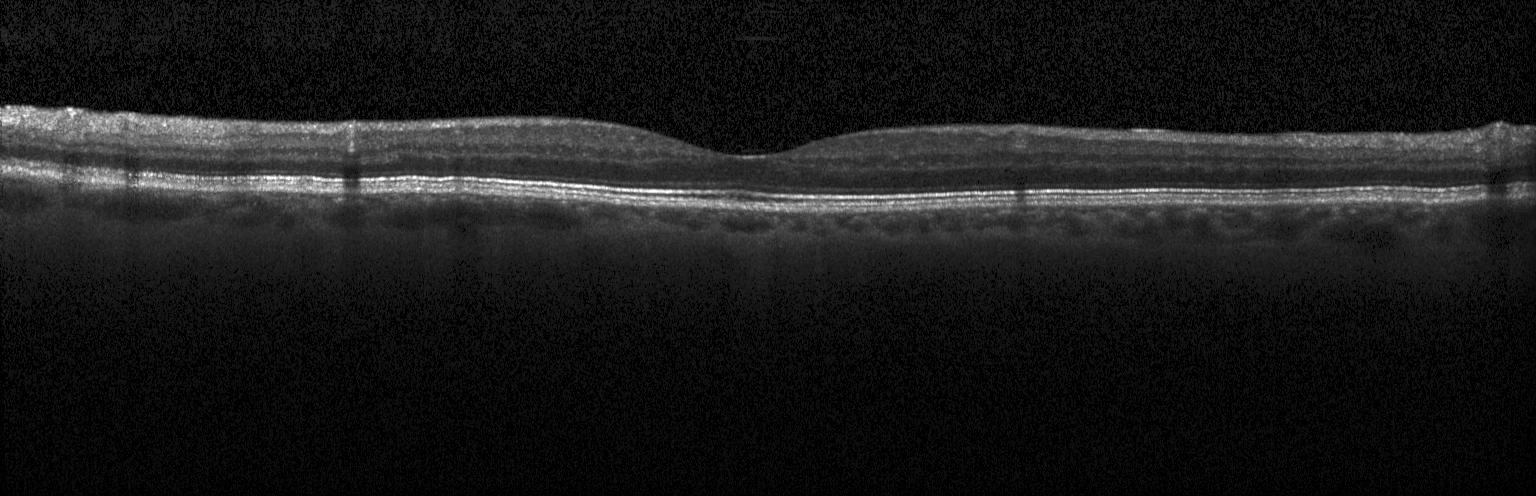
Macular OCT: no evidence of choroidal neovascularization, diabetic macular edema, or drusen.